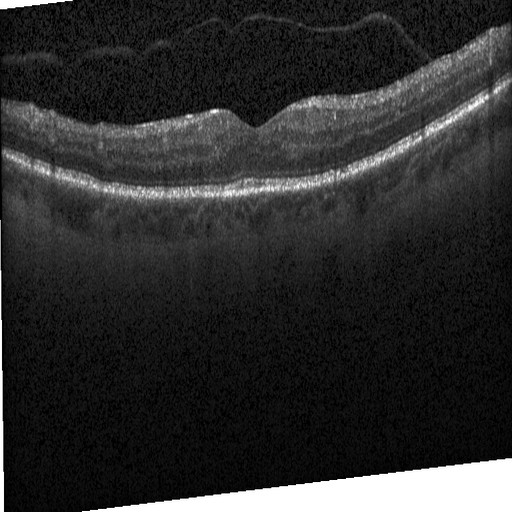
Diabetic macular edema (DME).